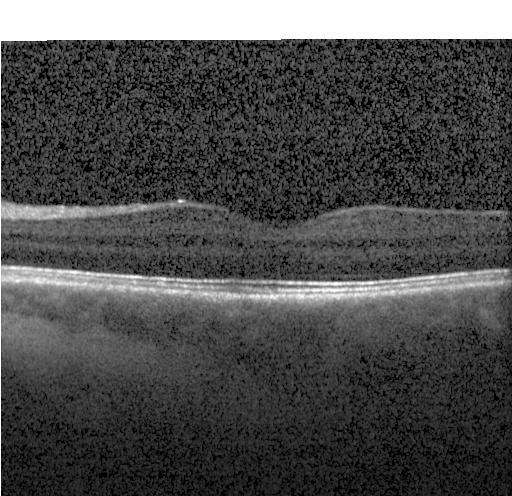
Retinal OCT cross-section showing no evidence of CNV, DME, or drusen.